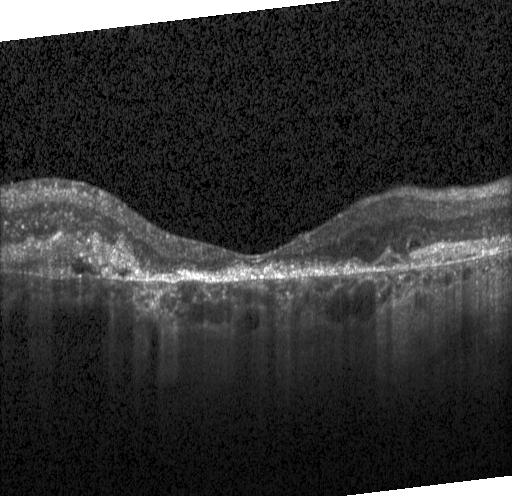 Finding: choroidal neovascularization.